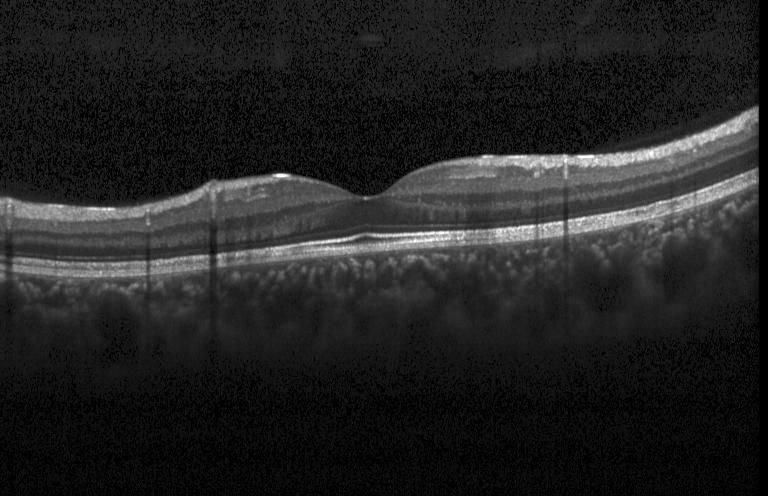
Impression: no CNV, no DME, and no drusen.